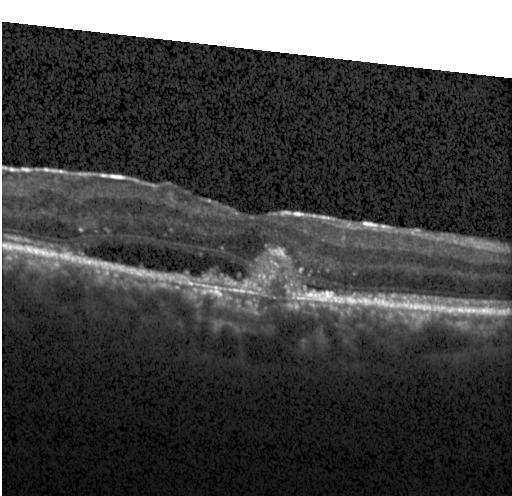
OCT finding: choroidal neovascularization.